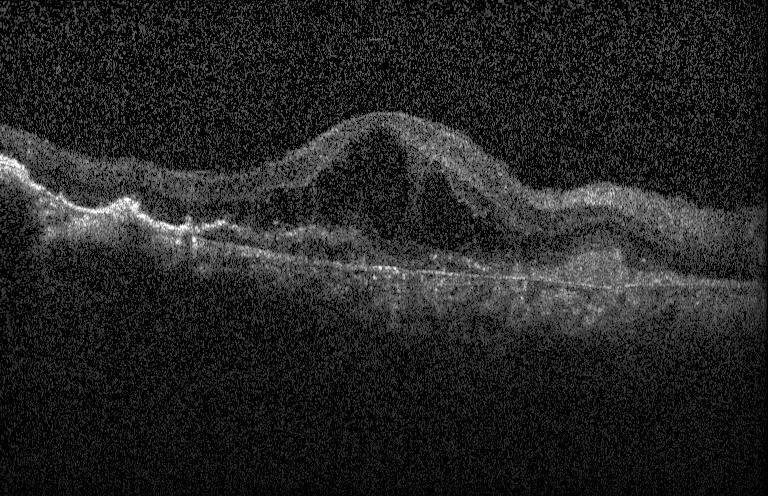
Optical coherence tomography scan.
Diagnosis: a choroidal neovascular membrane.